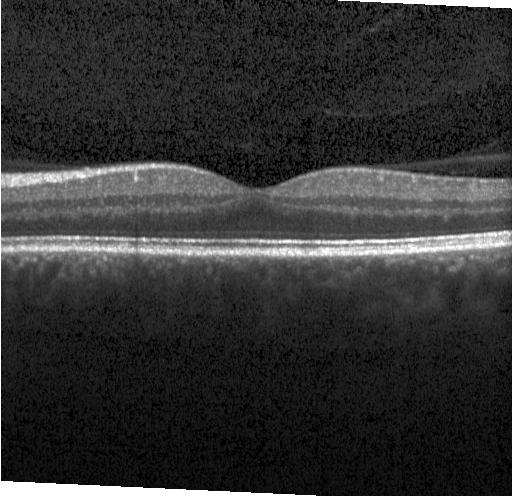

Optical coherence tomography scan · spectral-domain optical coherence tomography · acquired on a Heidelberg Spectralis · centered on the fovea
OCT finding: no choroidal neovascularization, no diabetic macular edema, and no drusen.